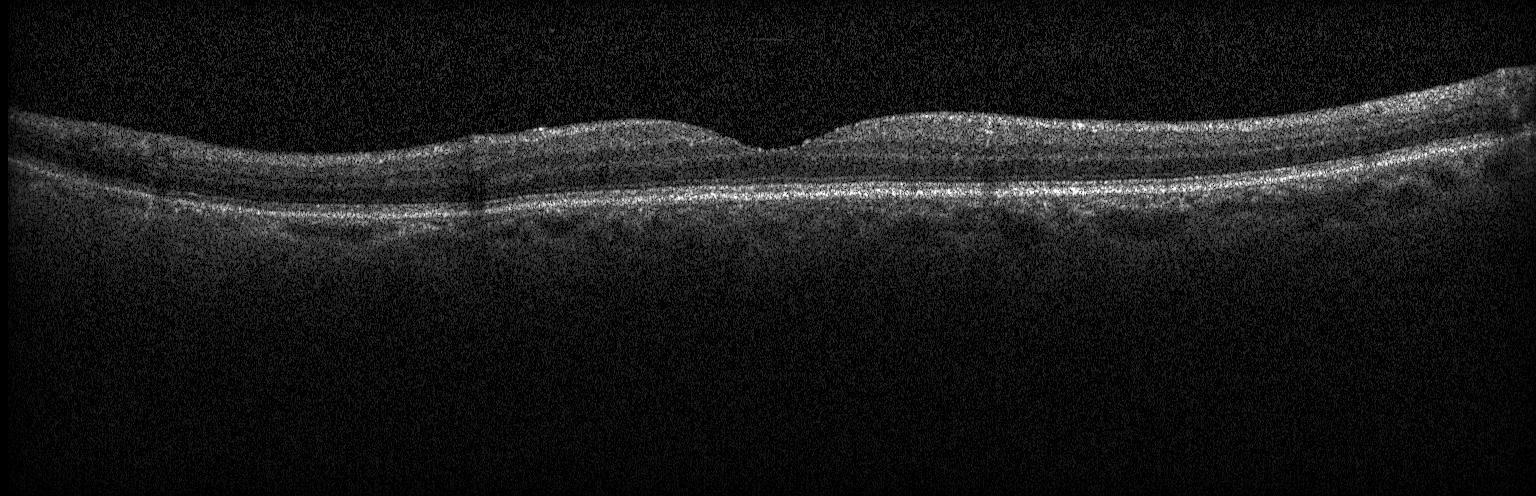
Optical coherence tomography scan · centered on the fovea · Heidelberg Spectralis OCT system
Finding: no evidence of choroidal neovascularization, diabetic macular edema, or drusen.